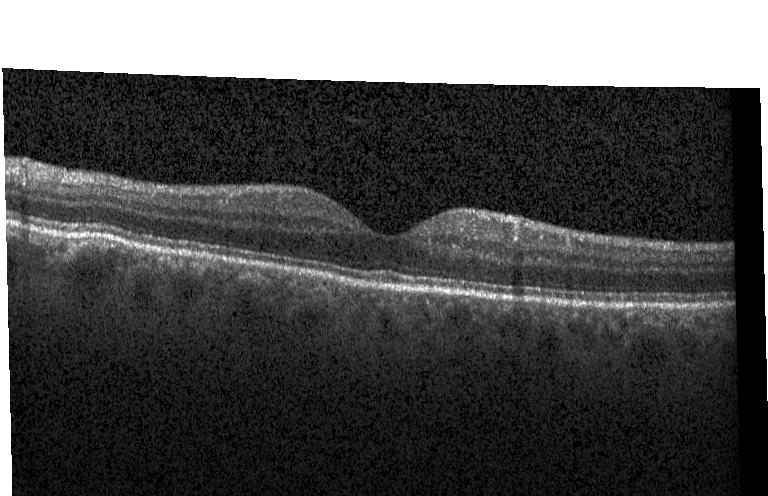
No evidence of choroidal neovascularization, diabetic macular edema, or drusen.